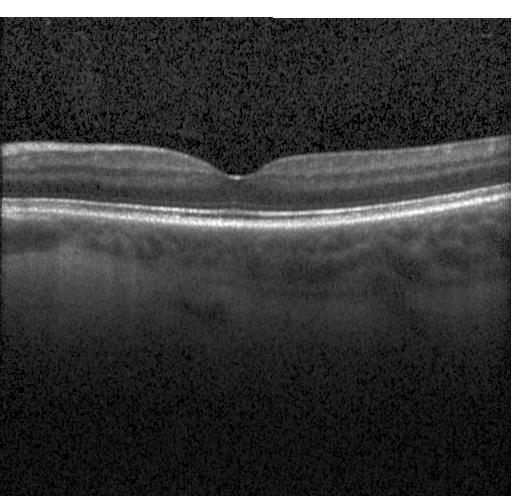 Optical coherence tomography scan, spectral-domain optical coherence tomography, Heidelberg Spectralis OCT system
Diagnosis: no evidence of choroidal neovascularization, diabetic macular edema, or drusen.